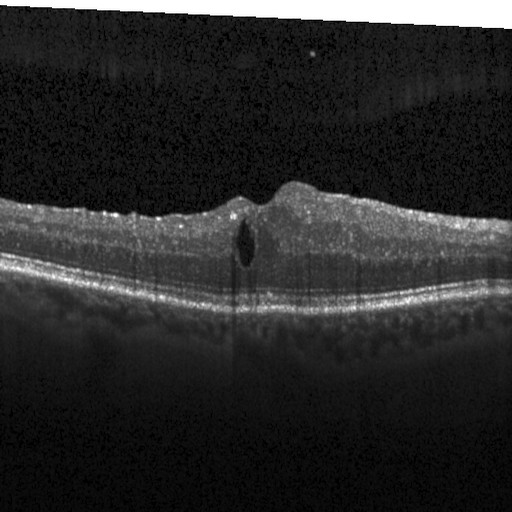 Spectral-domain optical coherence tomography, instrument: Heidelberg Spectralis, OCT B-scan, through the macula — Macular OCT: diabetic macular edema (DME).